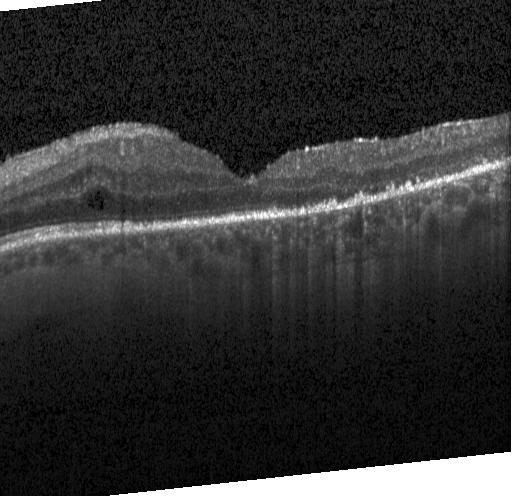 Spectral-domain OCT, OCT B-scan
Finding: diabetic macular edema.